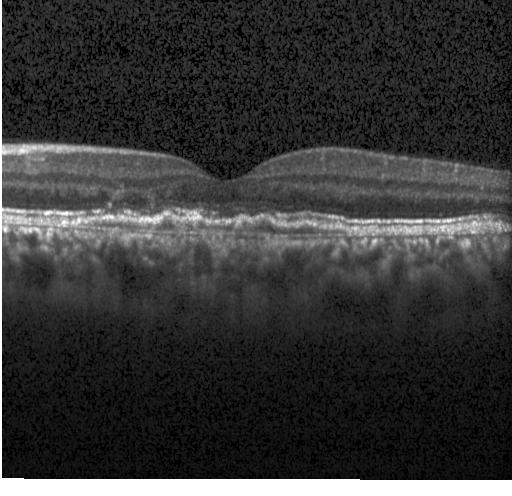
Spectral-domain OCT B-scan: CNV.